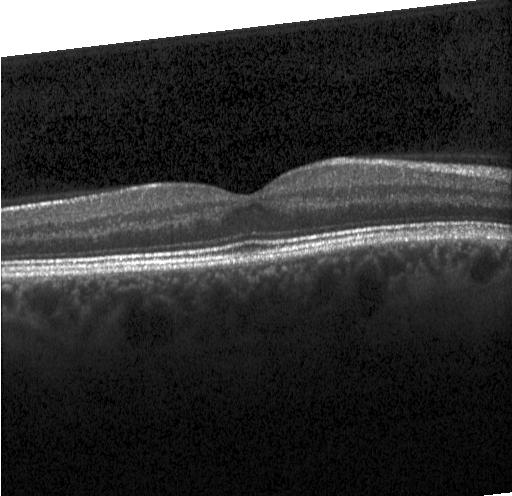 Optical coherence tomography B-scan.
Diagnosis: neither CNV, DME, nor drusen.